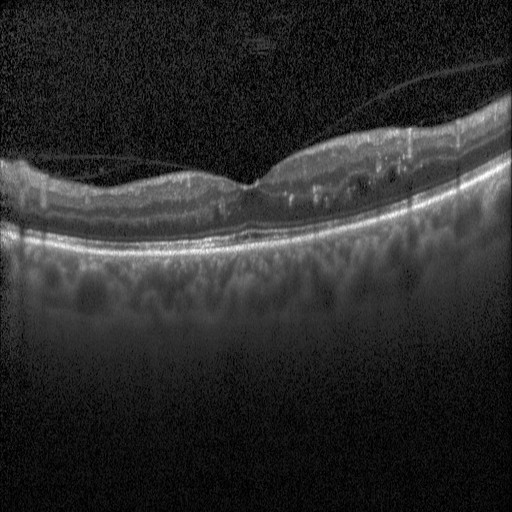

Retinal OCT B-scan; spectral-domain OCT; instrument: Heidelberg Spectralis. OCT finding: DME.